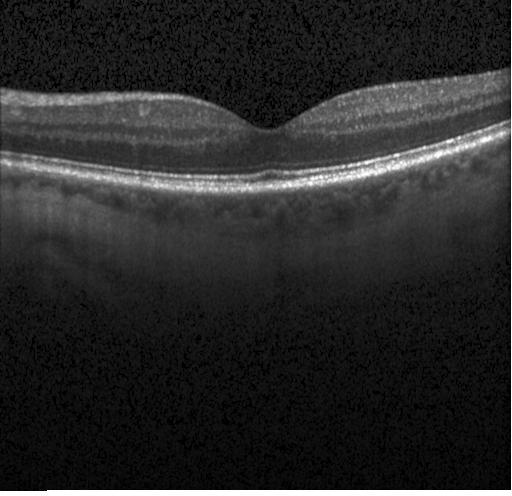

This B-scan demonstrates no CNV, no DME, and no drusen.